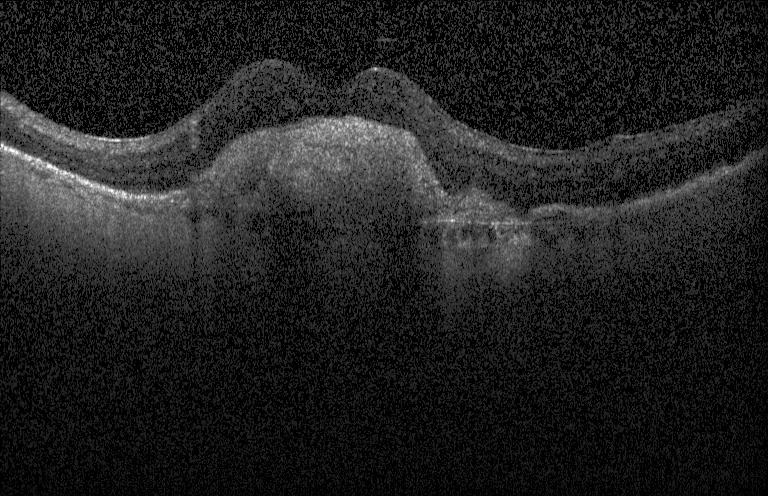

SD-OCT; centered on the fovea; retinal OCT cross-section.
This B-scan demonstrates CNV.